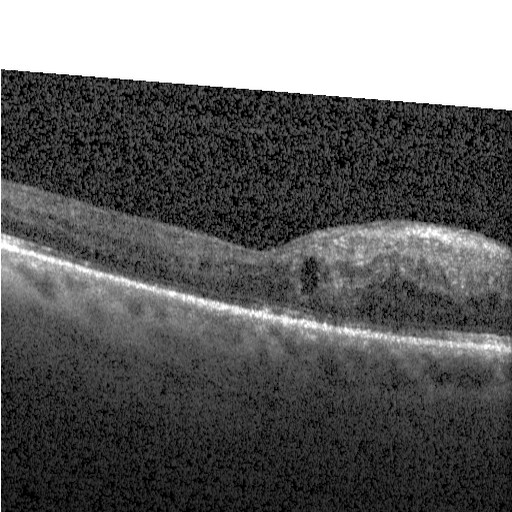
Optical coherence tomography scan, Heidelberg Spectralis
This B-scan demonstrates diabetic macular edema.